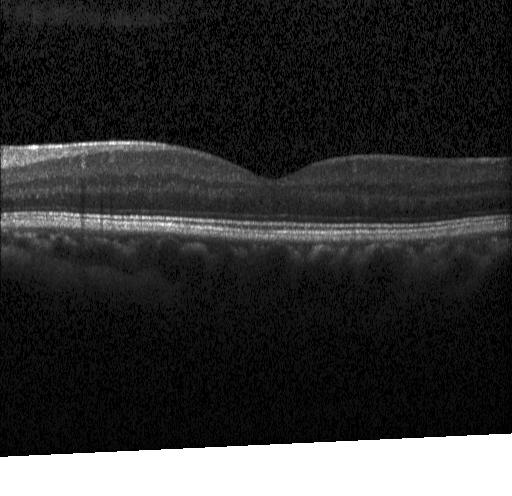

OCT scan showing no evidence of choroidal neovascularization, diabetic macular edema, or drusen.